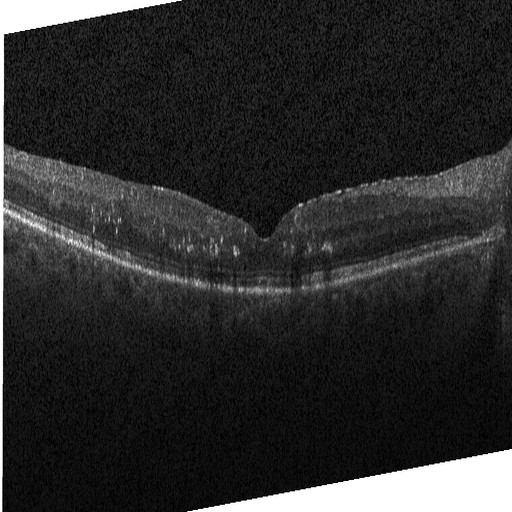
Finding: DME.